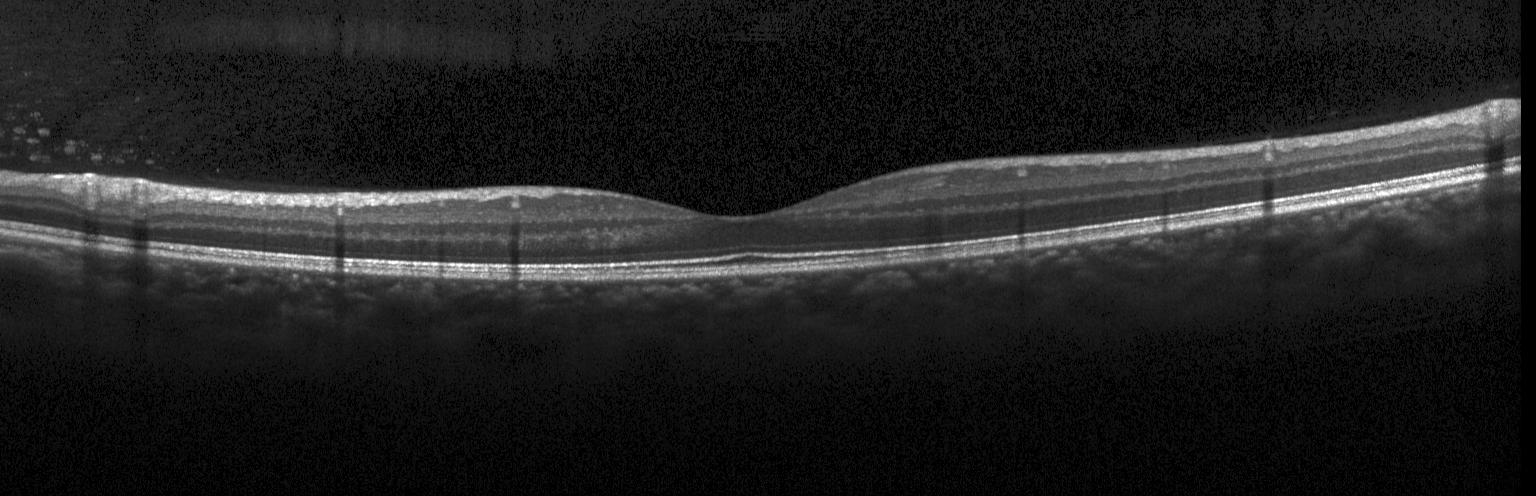

Retinal OCT cross-section · through the macula
Impression: no CNV, DME, or drusen.